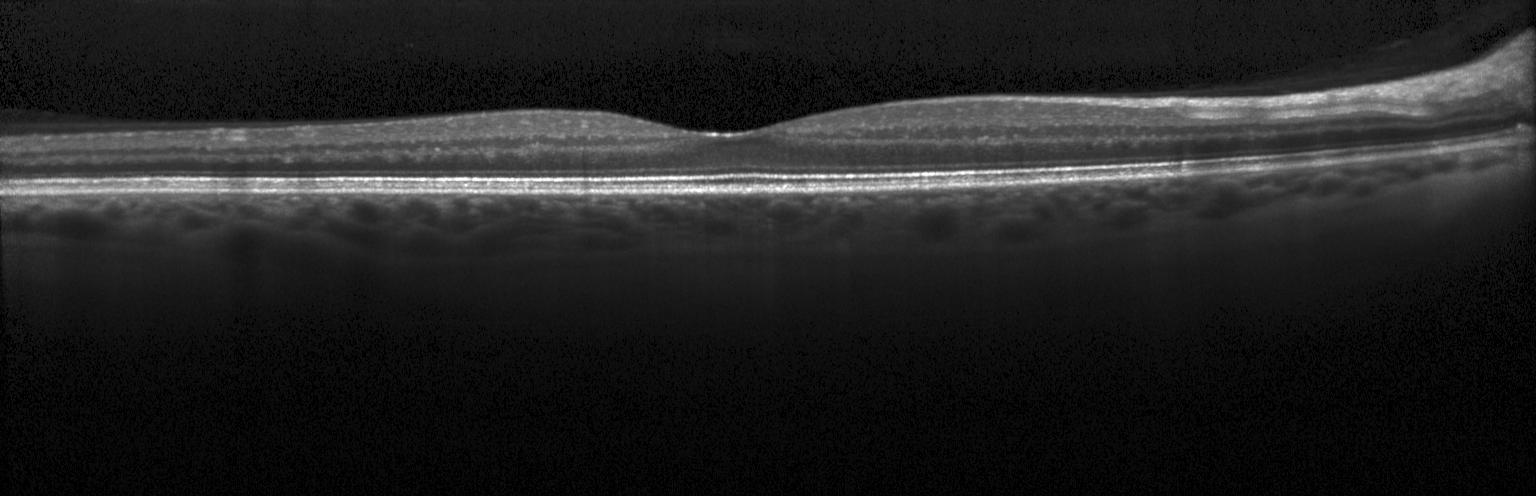

OCT B-scan, macular scan — Impression: no choroidal neovascularization, diabetic macular edema, or drusen.